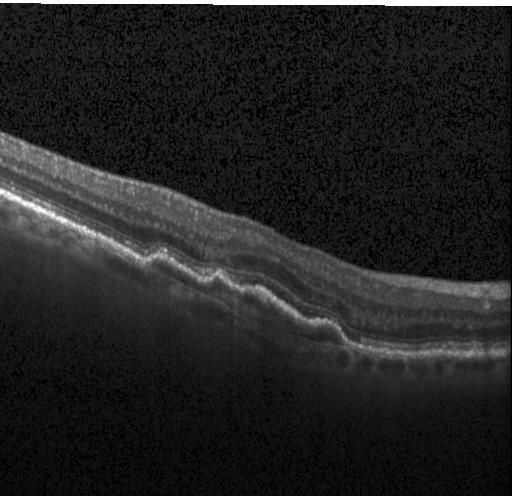

A choroidal neovascular membrane.